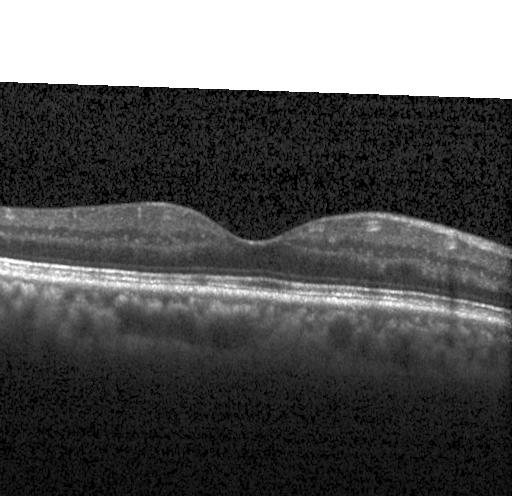 Acquired on a Heidelberg Spectralis, spectral-domain OCT, optical coherence tomography B-scan.
Diagnosis: no evidence of choroidal neovascularization, diabetic macular edema, or drusen.